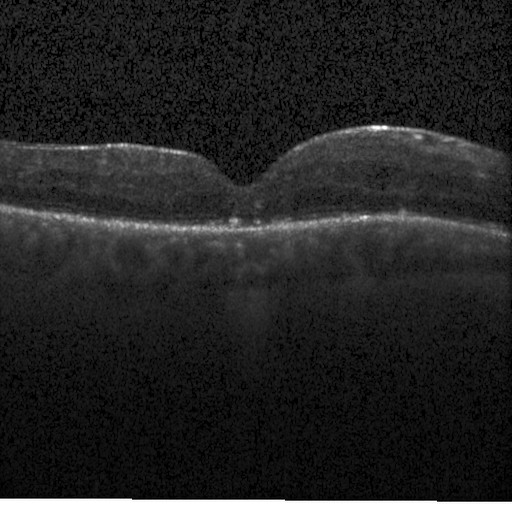

Acquired on a Heidelberg Spectralis · optical coherence tomography B-scan.
Impression: diabetic macular edema.